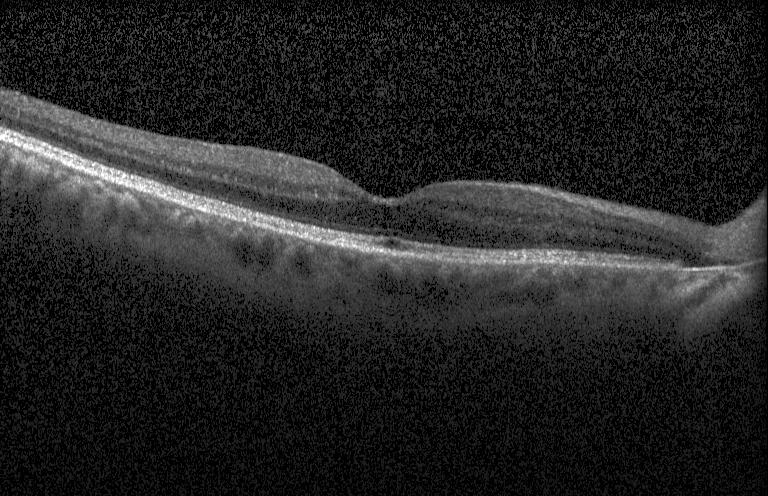
Fovea-centered, retinal OCT B-scan, Heidelberg Spectralis OCT system — Impression: no CNV, DME, or drusen.